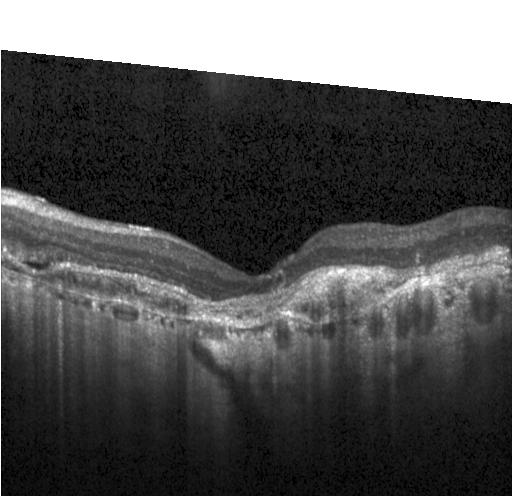

Spectral-domain OCT B-scan: a choroidal neovascular membrane.